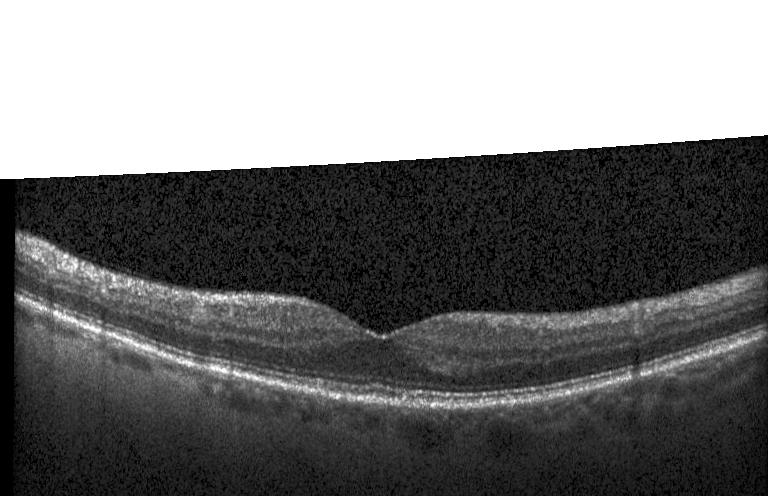 OCT B-scan — Neither choroidal neovascularization, diabetic macular edema, nor drusen.